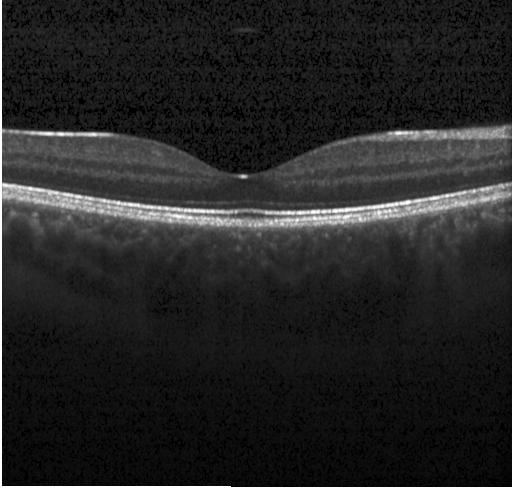
OCT finding: neither CNV, DME, nor drusen.